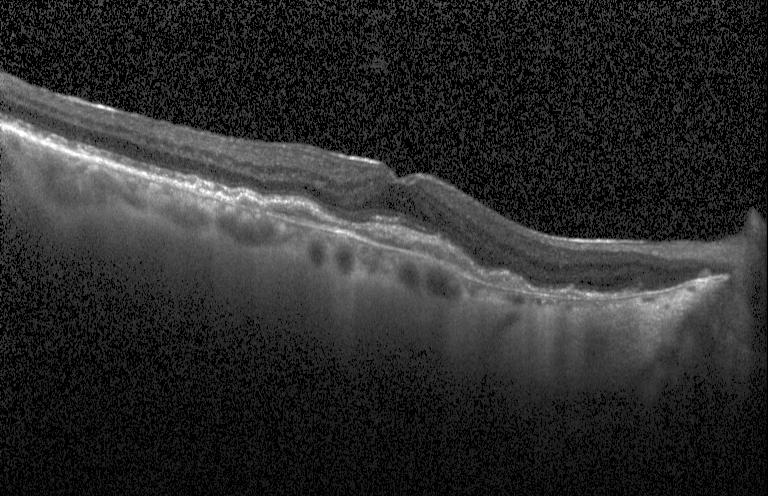

Macular OCT demonstrating a choroidal neovascular membrane.